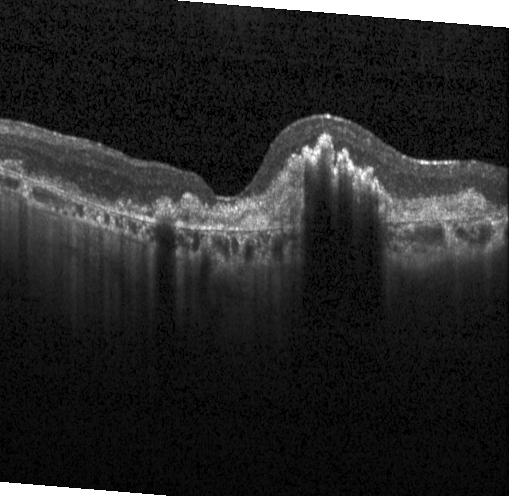

This B-scan demonstrates a choroidal neovascular membrane.